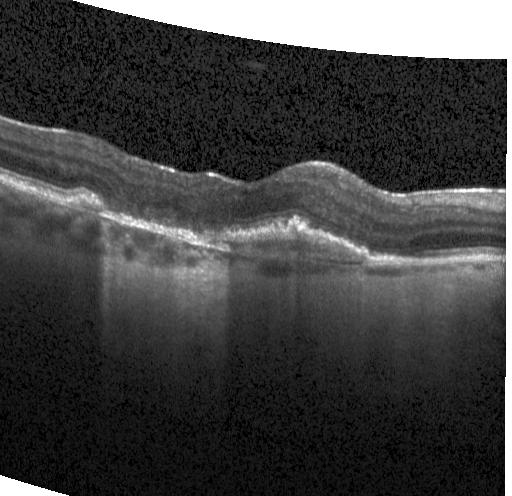

A choroidal neovascular membrane.